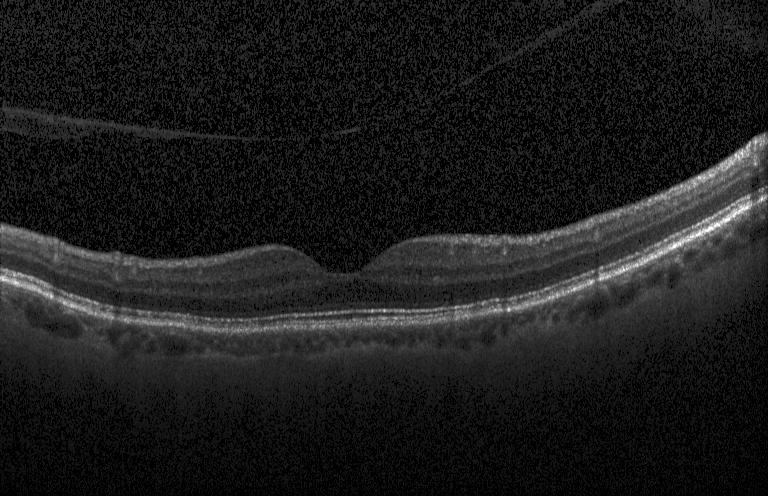

OCT B-scan. Spectral-domain optical coherence tomography. Instrument: Heidelberg Spectralis. Centered on the fovea. OCT finding: neither CNV, DME, nor drusen.